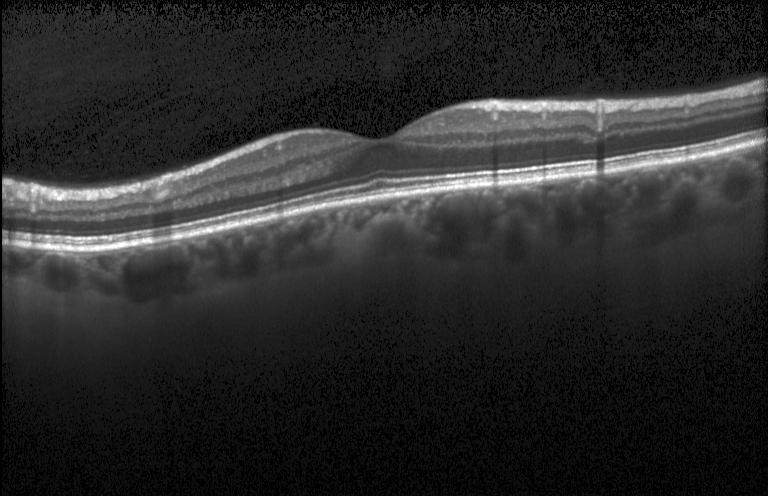 Retinal OCT B-scan. SD-OCT. Macular scan.
This B-scan demonstrates no CNV, no DME, and no drusen.